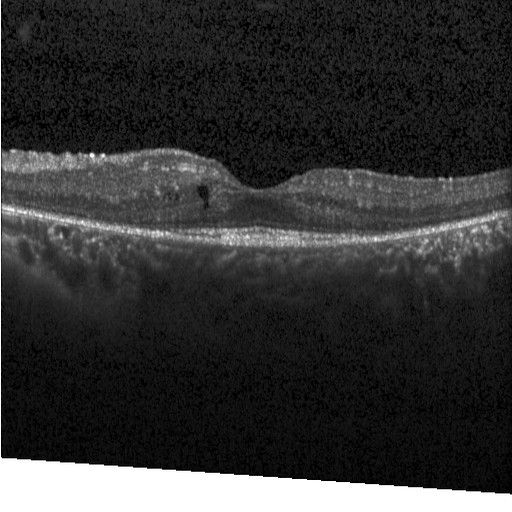

Finding: diabetic macular edema (DME).